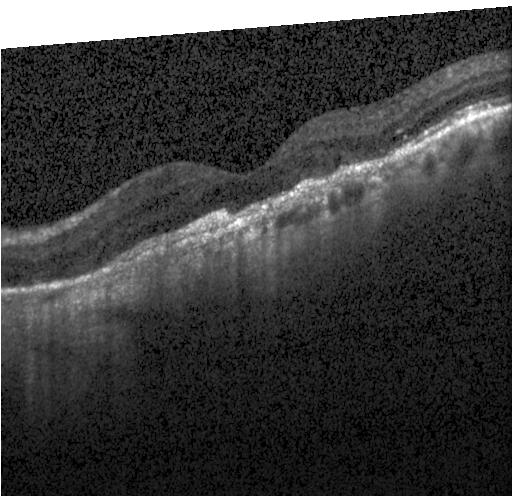
A choroidal neovascular membrane.